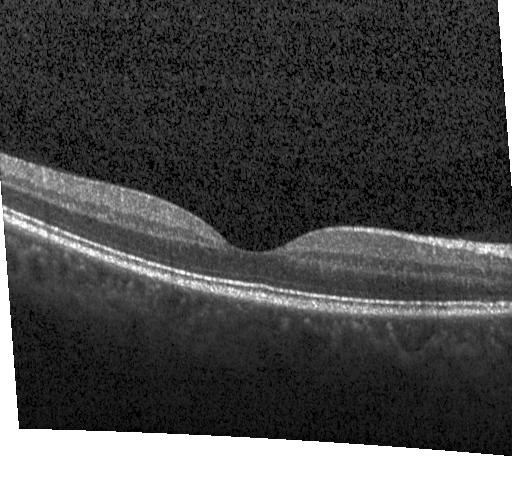
OCT B-scan. SD-OCT. Centered on the fovea — Impression: no choroidal neovascularization, diabetic macular edema, or drusen.